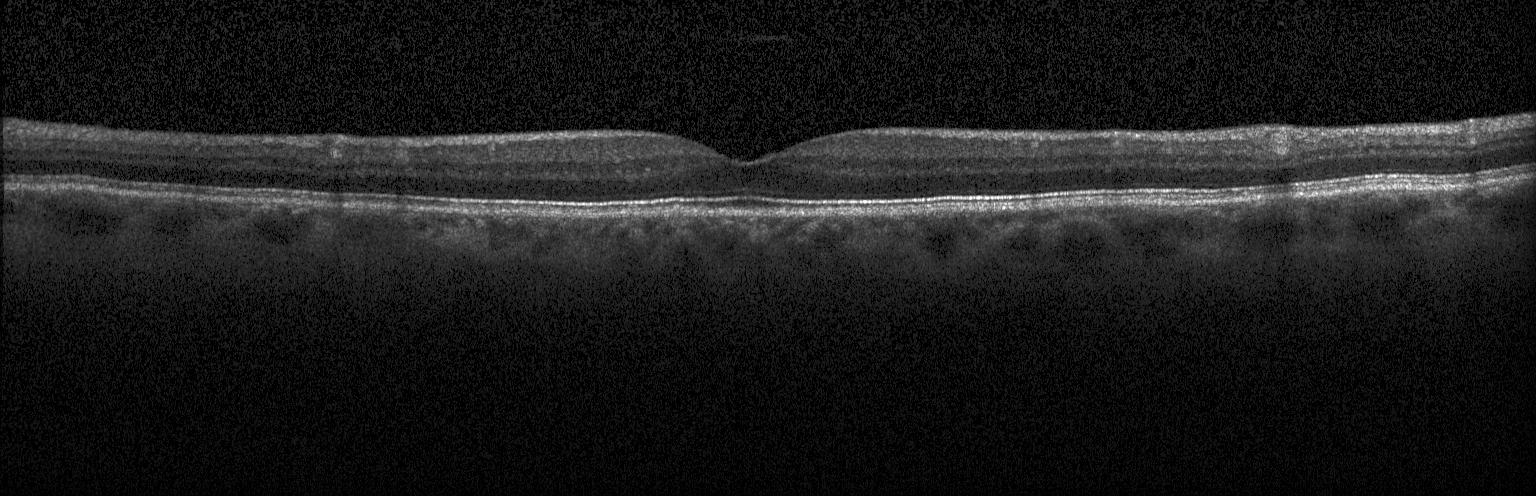

Diagnosis: no choroidal neovascularization, no diabetic macular edema, and no drusen.